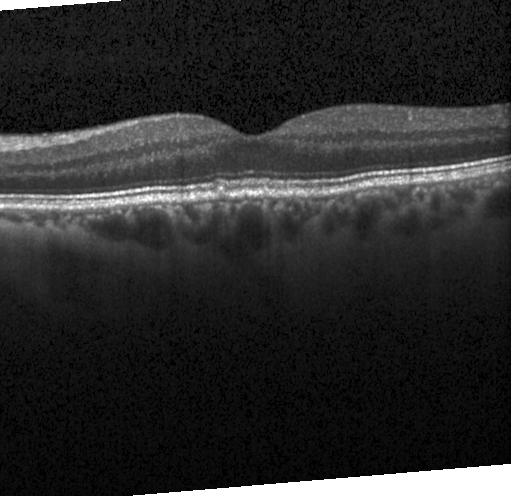 Spectral-domain optical coherence tomography, fovea-centered, optical coherence tomography scan — Diagnosis: sub-RPE drusenoid deposits.